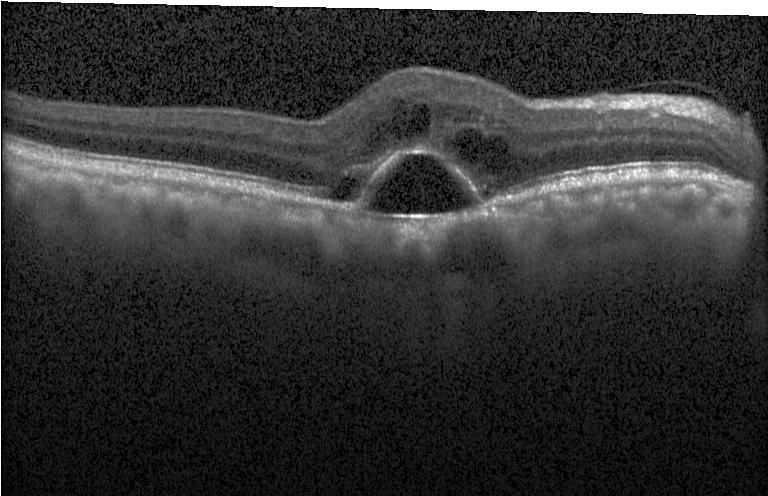 The scan shows CNV.